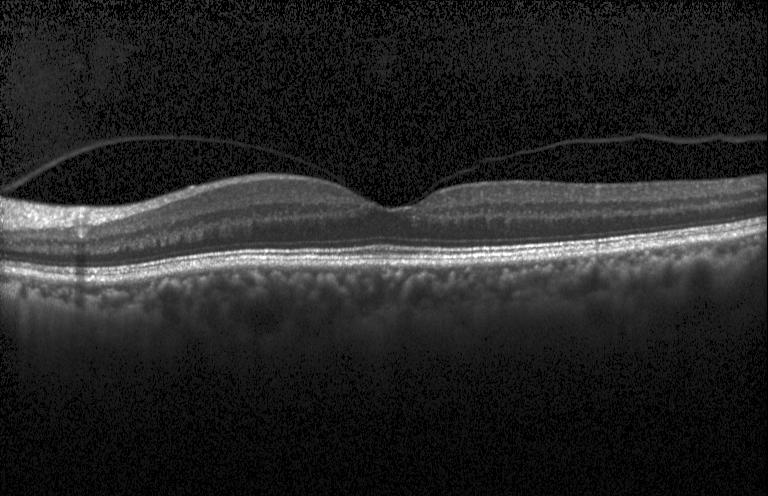 Optical coherence tomography B-scan, spectral-domain optical coherence tomography, macular scan
This B-scan demonstrates no evidence of choroidal neovascularization, diabetic macular edema, or drusen.